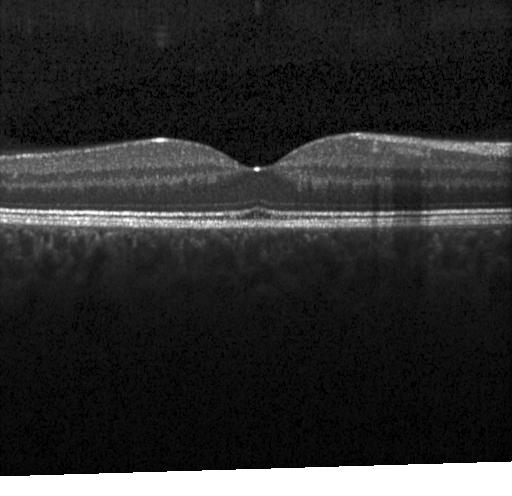
Spectral-domain OCT. Acquired on a Heidelberg Spectralis. Centered on the fovea. OCT B-scan
Diagnosis: no evidence of choroidal neovascularization, diabetic macular edema, or drusen.